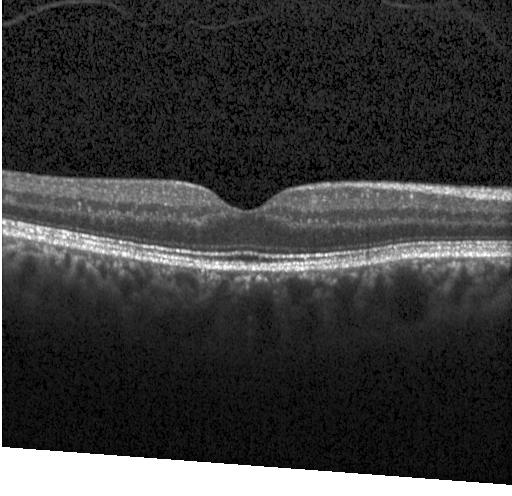
Spectral-domain OCT B-scan: no evidence of choroidal neovascularization, diabetic macular edema, or drusen.